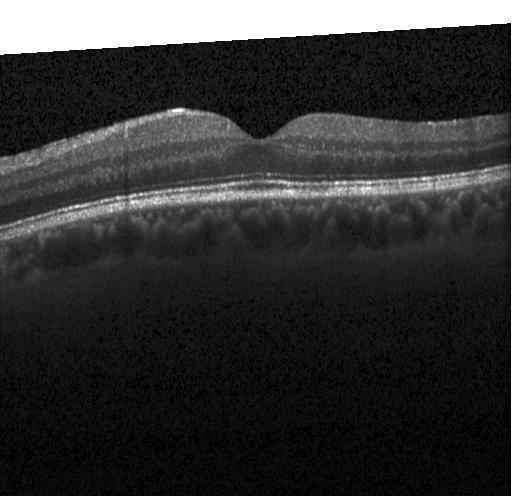
No evidence of choroidal neovascularization, diabetic macular edema, or drusen.